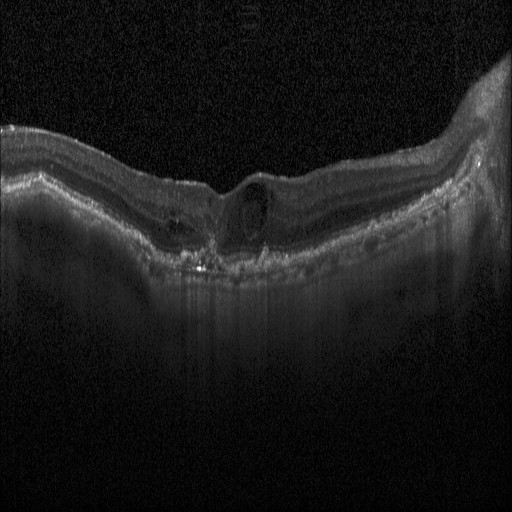 Heidelberg Spectralis OCT system. Retinal OCT B-scan
Impression: DME.